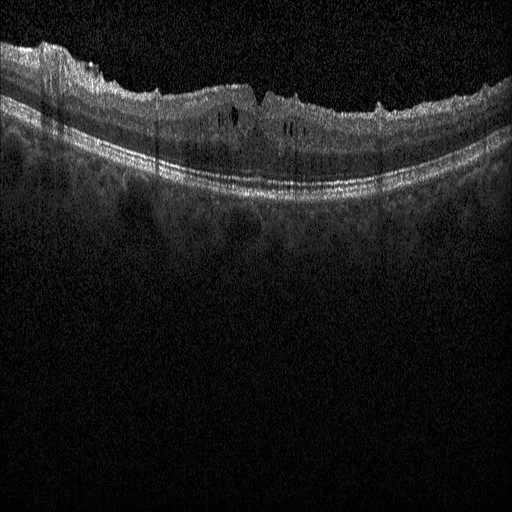

Impression: diabetic macular edema (DME).